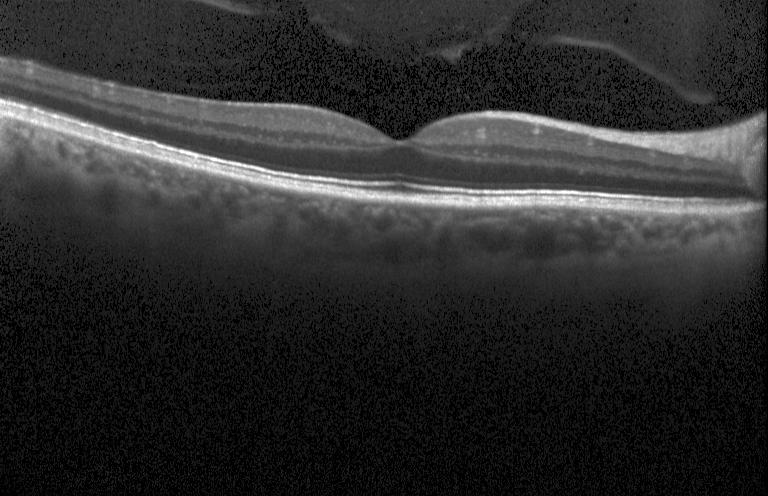
Optical coherence tomography scan; fovea-centered; spectral-domain optical coherence tomography; Heidelberg Spectralis — No evidence of choroidal neovascularization, diabetic macular edema, or drusen.